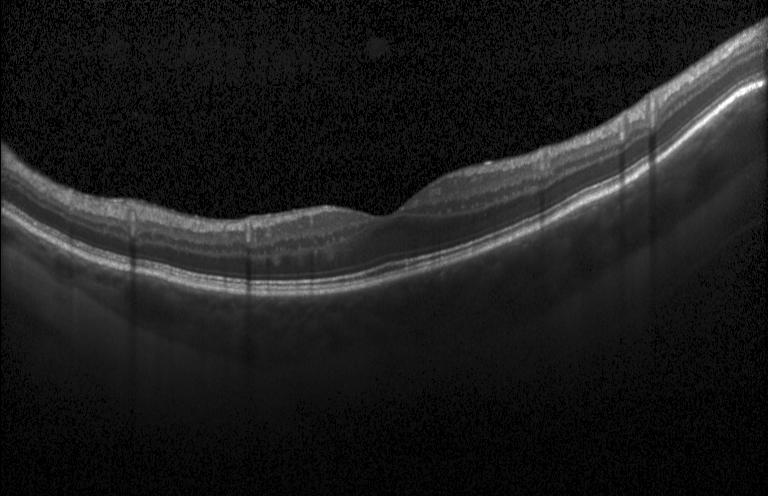
Heidelberg Spectralis OCT system, optical coherence tomography B-scan, macular scan.
The scan shows neither choroidal neovascularization, diabetic macular edema, nor drusen.